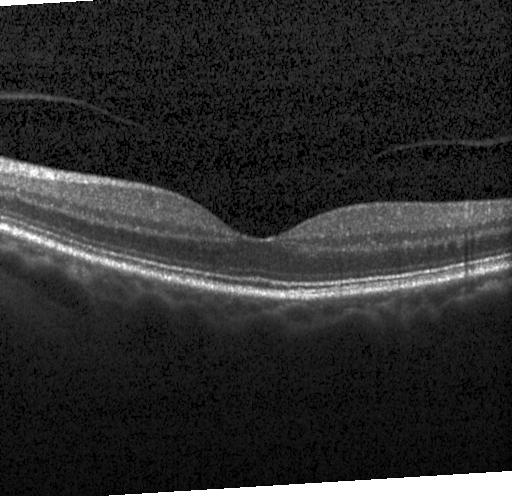

Macular OCT demonstrating no choroidal neovascularization, no diabetic macular edema, and no drusen.